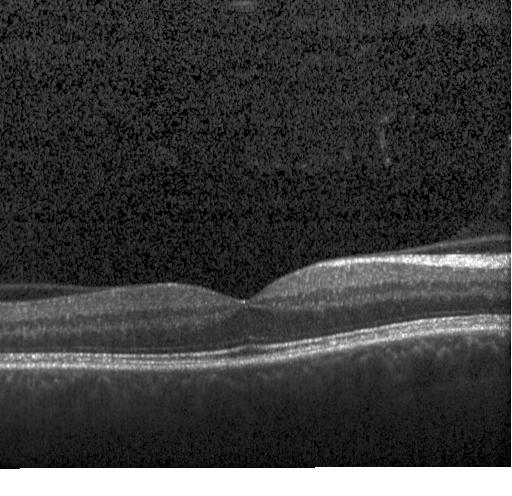

Assessment: no choroidal neovascularization, no diabetic macular edema, and no drusen.